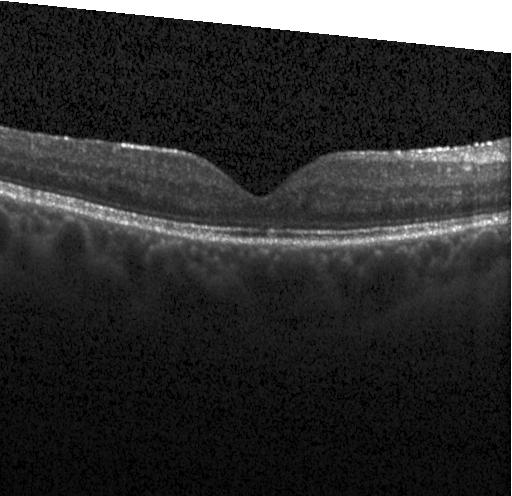

Spectral-domain OCT. Optical coherence tomography B-scan.
Finding: no evidence of CNV, DME, or drusen.